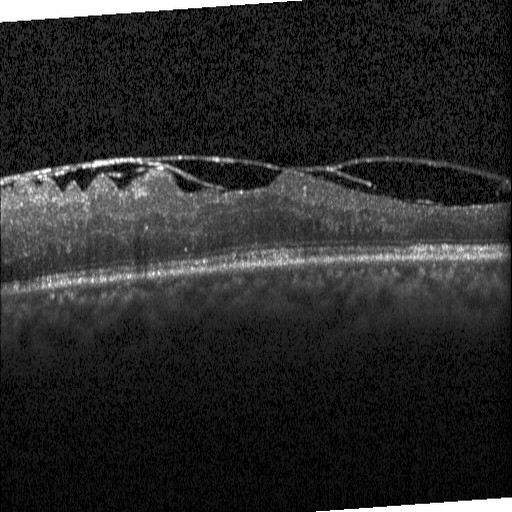
Optical coherence tomography B-scan · SD-OCT · acquired on a Heidelberg Spectralis · fovea-centered
Finding: diabetic macular edema.